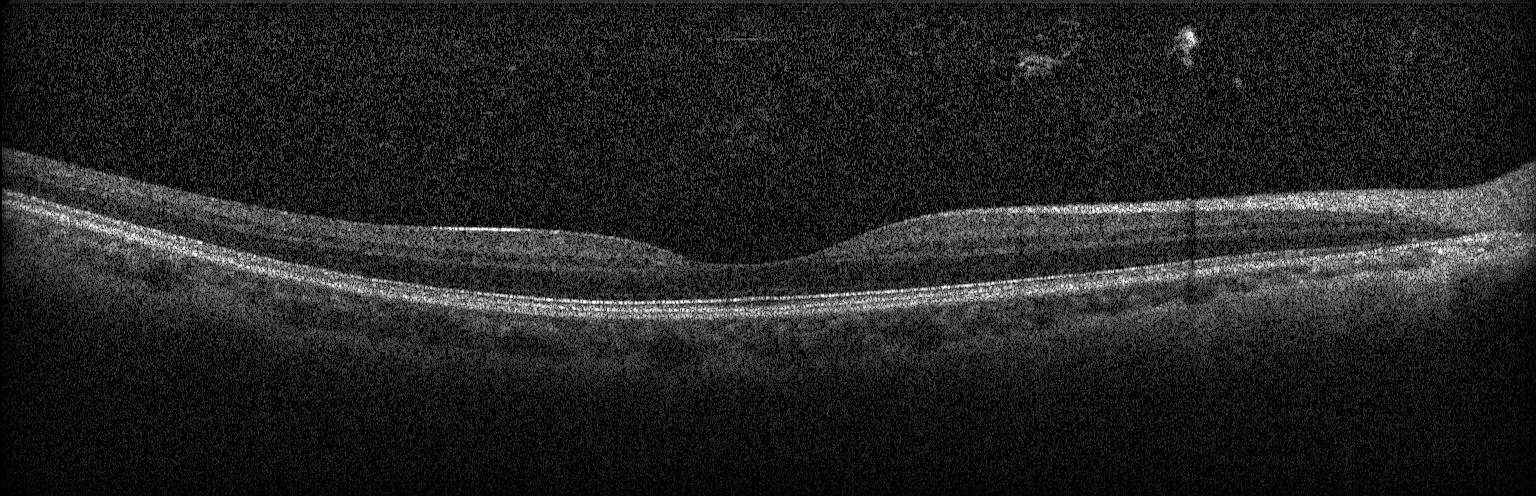 Retinal OCT cross-section — Diagnosis: no evidence of choroidal neovascularization, diabetic macular edema, or drusen.